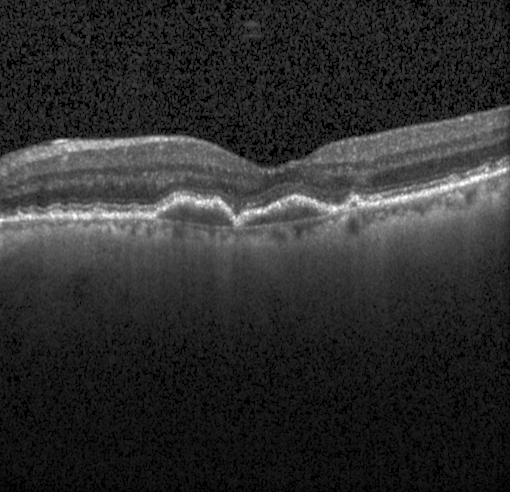 Spectral-domain optical coherence tomography; OCT B-scan; Heidelberg Spectralis; horizontal scan through the fovea.
Finding: a choroidal neovascular membrane.